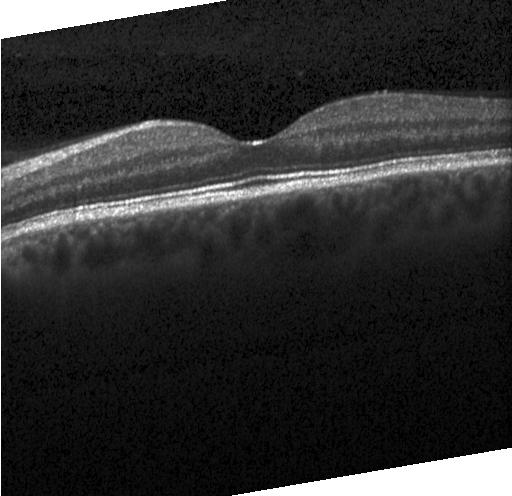

Fovea-centered, instrument: Heidelberg Spectralis, spectral-domain optical coherence tomography, OCT B-scan. Dx: neither CNV, DME, nor drusen.